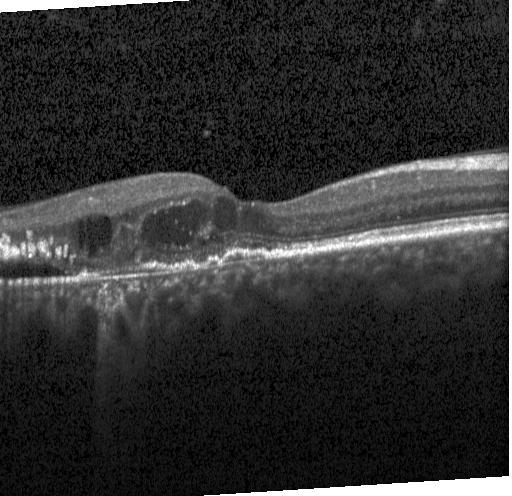

Macular OCT: choroidal neovascularization.